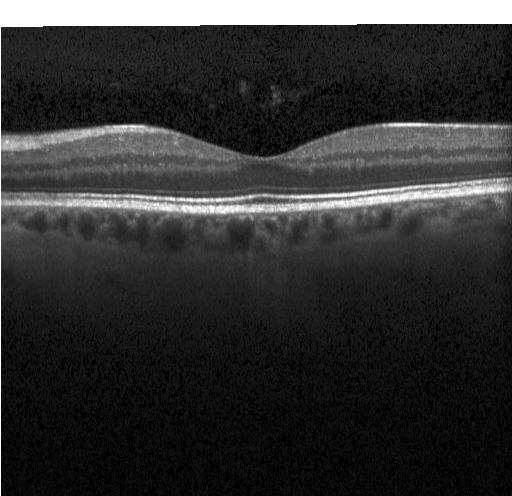

Fovea-centered; OCT B-scan; acquired on a Heidelberg Spectralis; spectral-domain optical coherence tomography. Dx: no evidence of CNV, DME, or drusen.